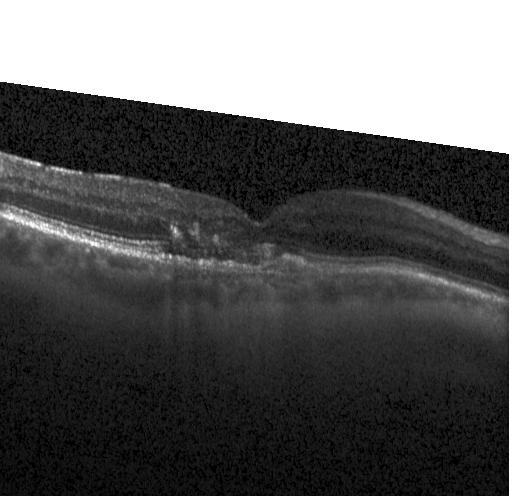

Retinal OCT cross-section; spectral-domain optical coherence tomography — Dx: a choroidal neovascular membrane.